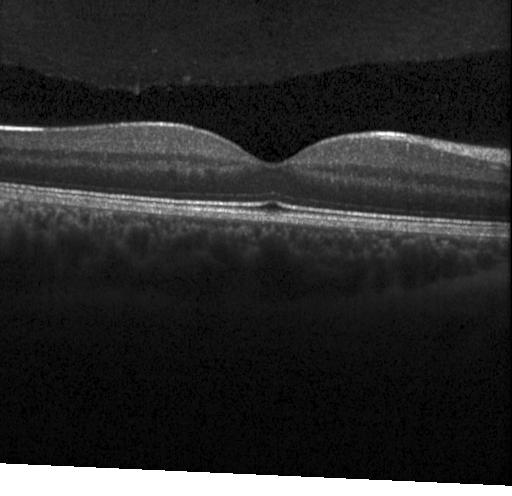 Instrument: Heidelberg Spectralis. Retinal OCT B-scan. Macular scan
Diagnosis: neither choroidal neovascularization, diabetic macular edema, nor drusen.